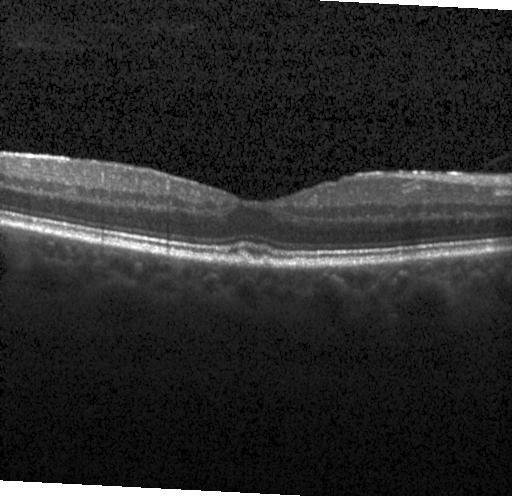 SD-OCT · retinal OCT B-scan — Dx: sub-RPE drusenoid deposits.